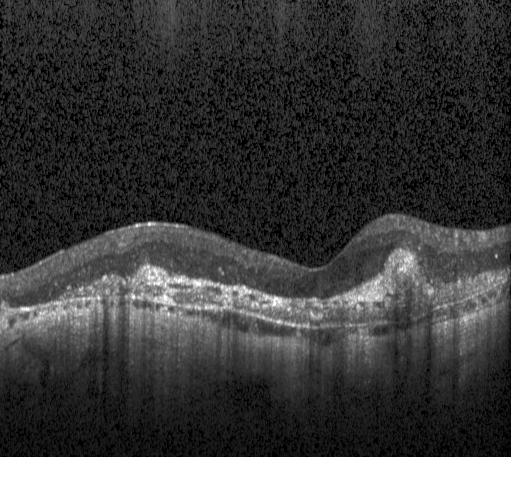
This B-scan demonstrates CNV.